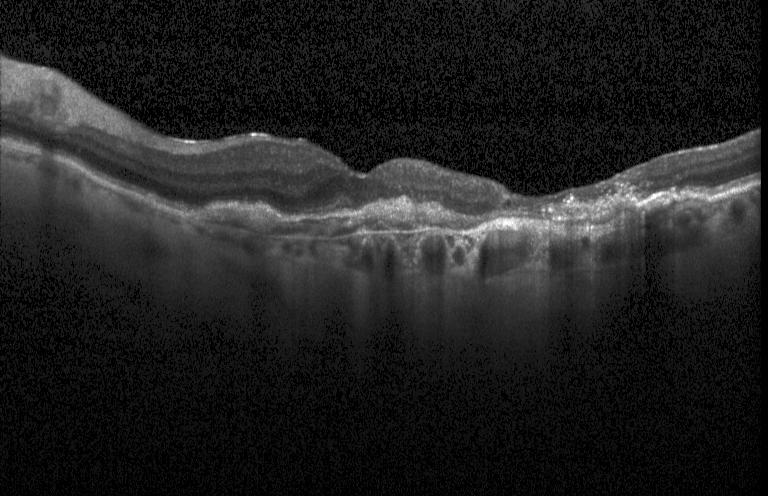 OCT finding: choroidal neovascularization (CNV).